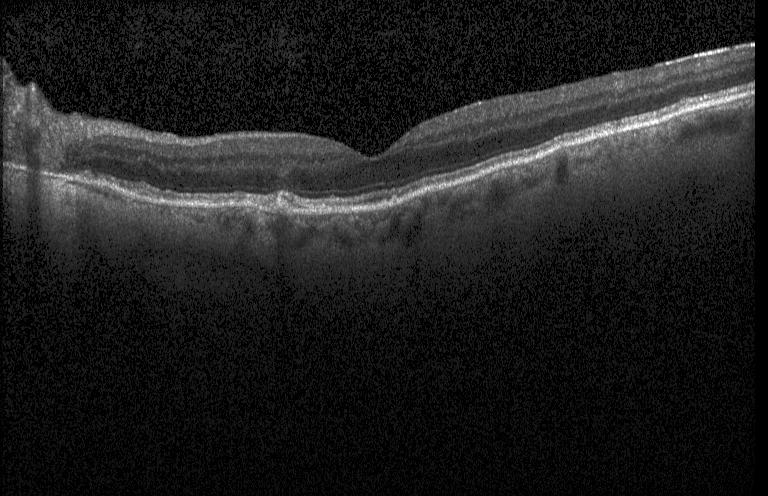 Optical coherence tomography B-scan · acquired on a Heidelberg Spectralis · spectral-domain optical coherence tomography · through the macula
The scan shows sub-RPE drusenoid deposits.